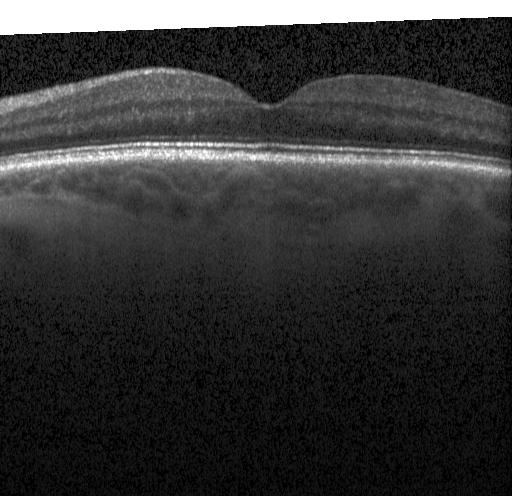
Optical coherence tomography B-scan. Finding: neither choroidal neovascularization, diabetic macular edema, nor drusen.